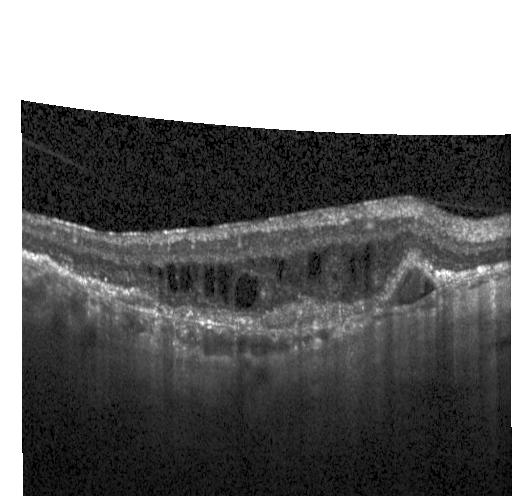
Optical coherence tomography scan, macular scan, spectral-domain OCT, Heidelberg Spectralis OCT system
Diagnosis: choroidal neovascularization (CNV).